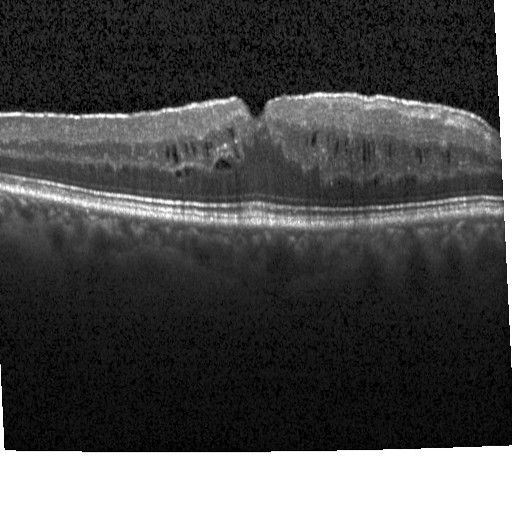
Through the macula. Retinal OCT B-scan
Macular OCT: DME.